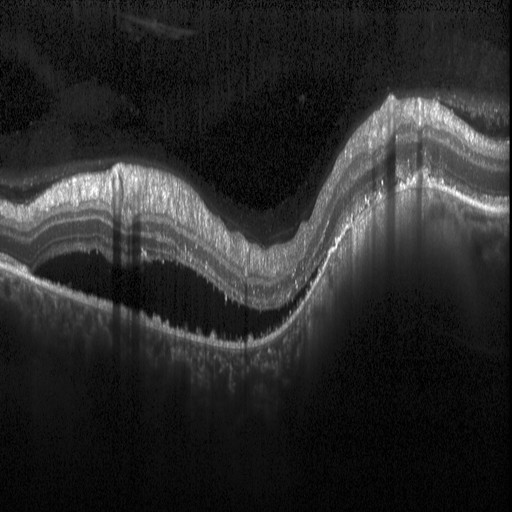 Fovea-centered. OCT B-scan. Spectral-domain OCT. Heidelberg Spectralis OCT system.
Diagnosis: DME.